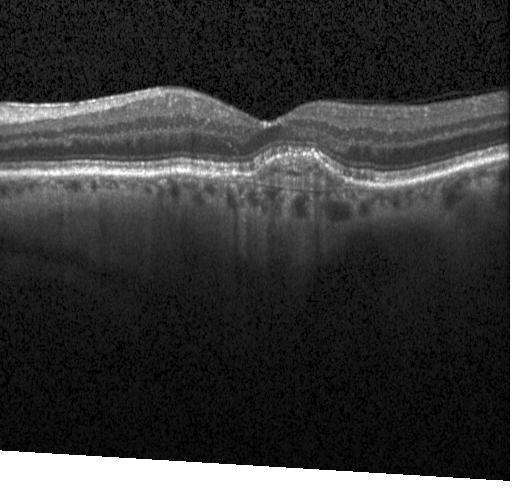

Acquired on a Heidelberg Spectralis. Optical coherence tomography scan — Impression: a choroidal neovascular membrane.